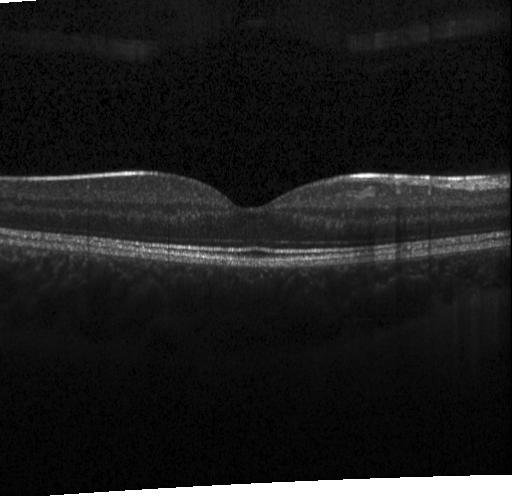
OCT B-scan; SD-OCT; horizontal scan through the fovea
Macular OCT: no choroidal neovascularization, diabetic macular edema, or drusen.